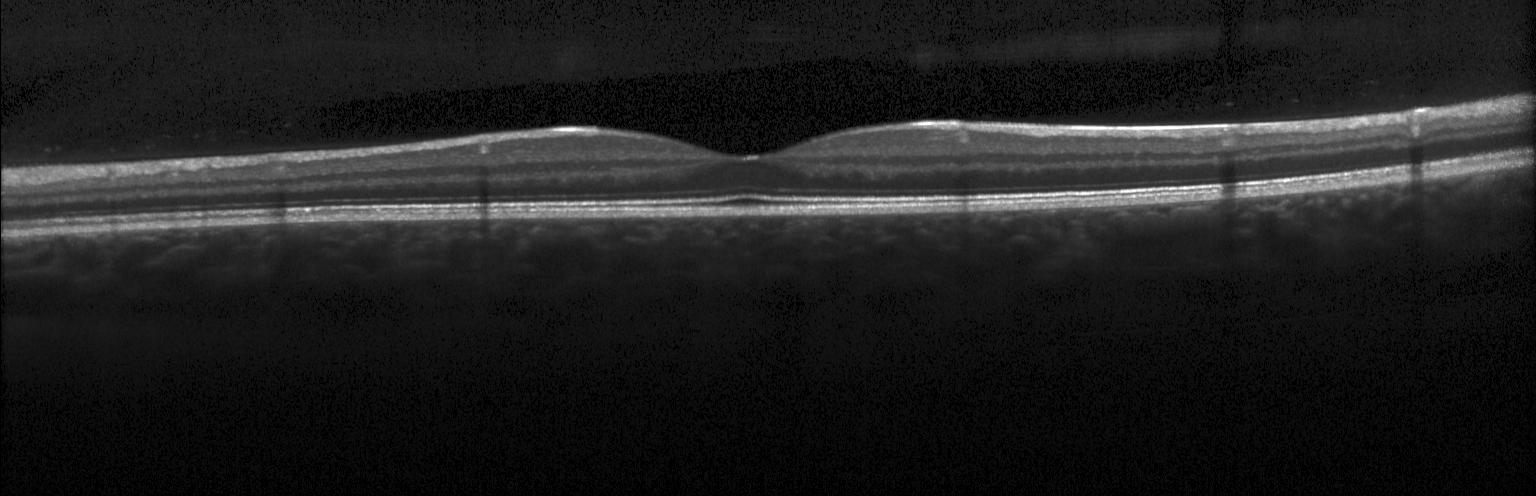
Spectral-domain OCT. OCT B-scan — Finding: no evidence of CNV, DME, or drusen.